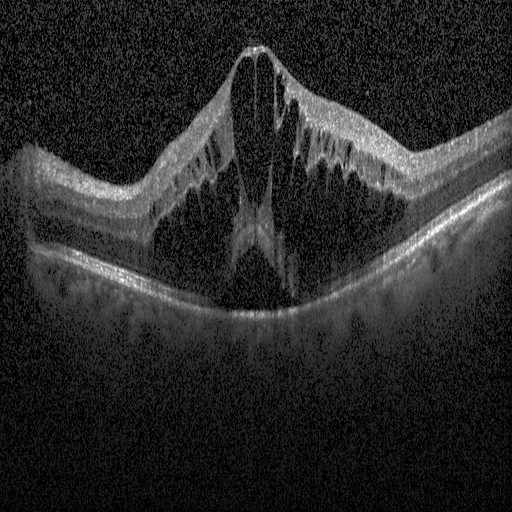

OCT finding: diabetic macular edema.